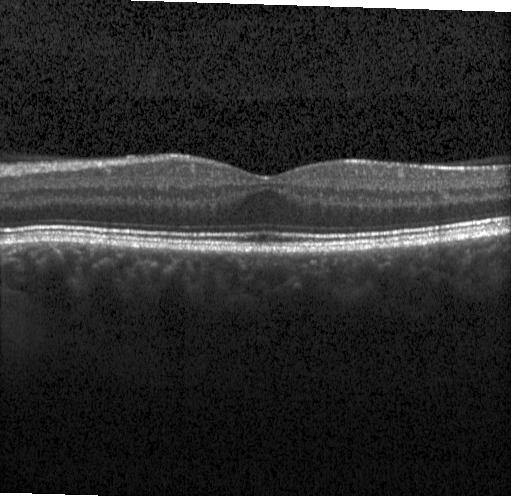
Diagnosis: no CNV, DME, or drusen.